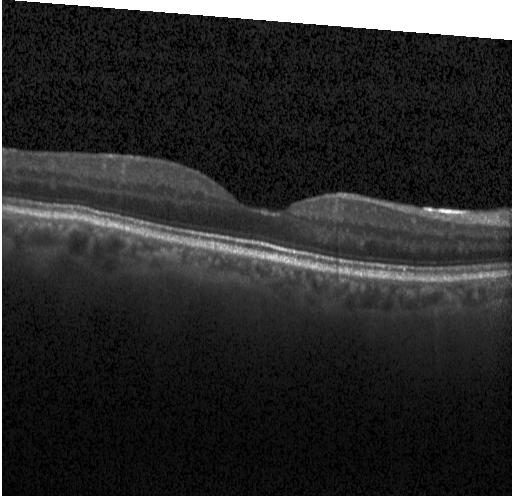
Spectral-domain optical coherence tomography; optical coherence tomography scan; horizontal scan through the fovea
Diagnosis: neither choroidal neovascularization, diabetic macular edema, nor drusen.